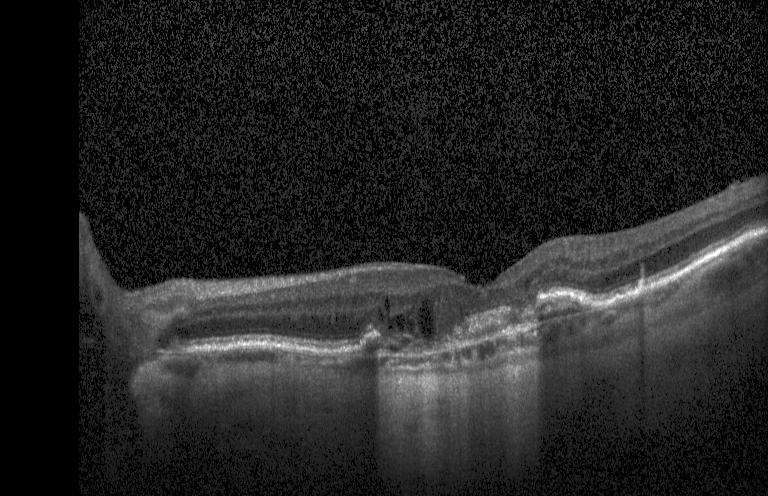

Optical coherence tomography scan; spectral-domain OCT. Finding: a choroidal neovascular membrane.